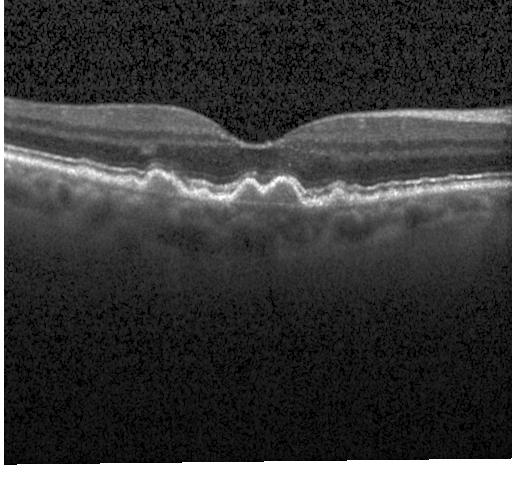

The scan shows drusen.